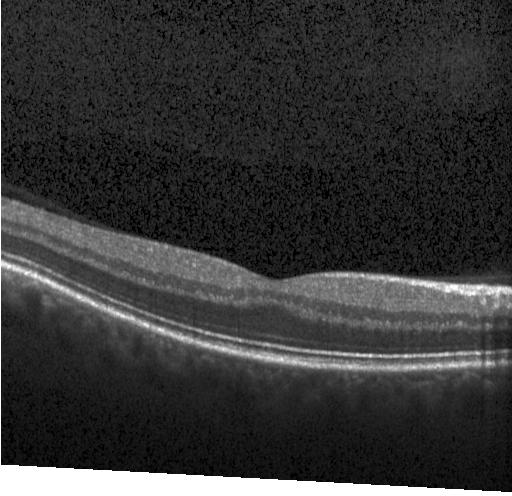
Spectral-domain optical coherence tomography; retinal OCT cross-section; Heidelberg Spectralis OCT system. No evidence of choroidal neovascularization, diabetic macular edema, or drusen.